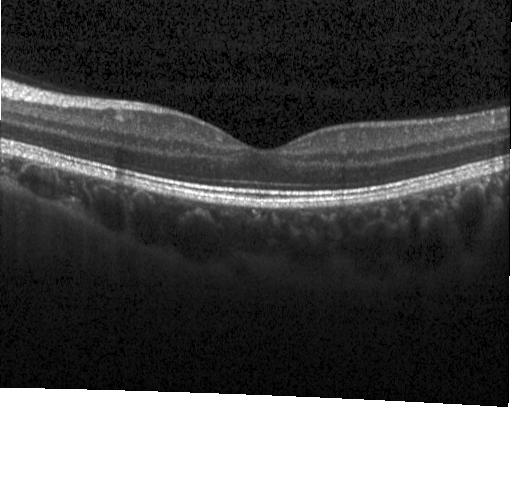
OCT scan showing no evidence of CNV, DME, or drusen.